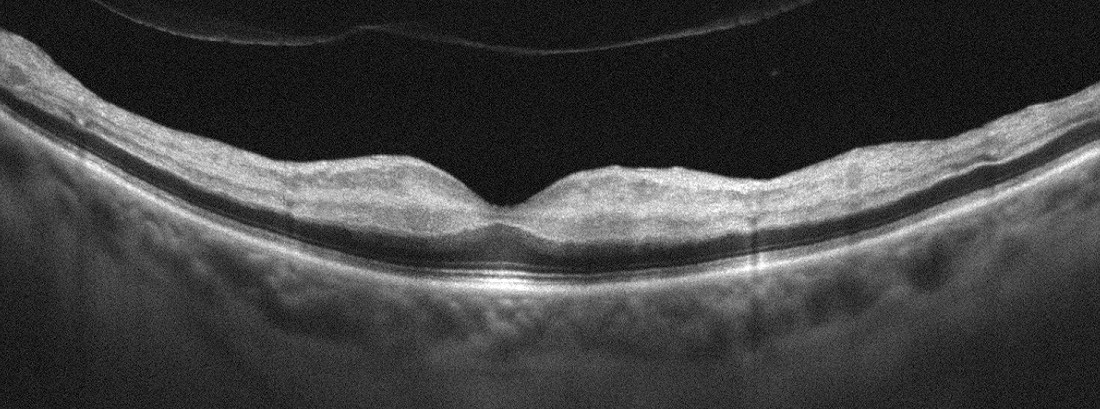
Optical coherence tomography B-scan.
Impression: retinal artery occlusion.